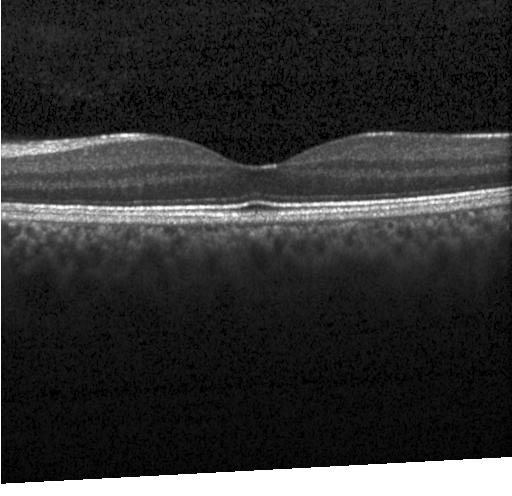
Optical coherence tomography scan, SD-OCT — Impression: no CNV, DME, or drusen.